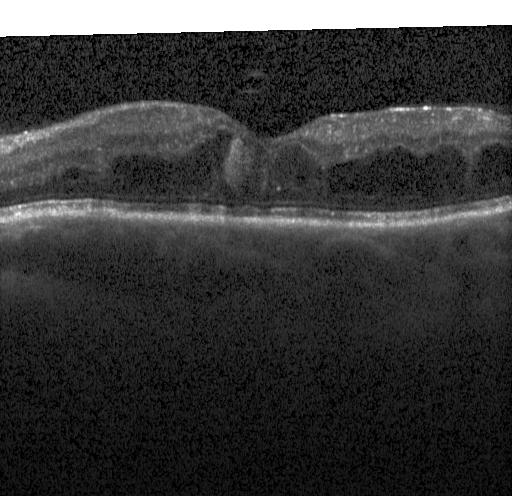

Finding: diabetic macular edema.